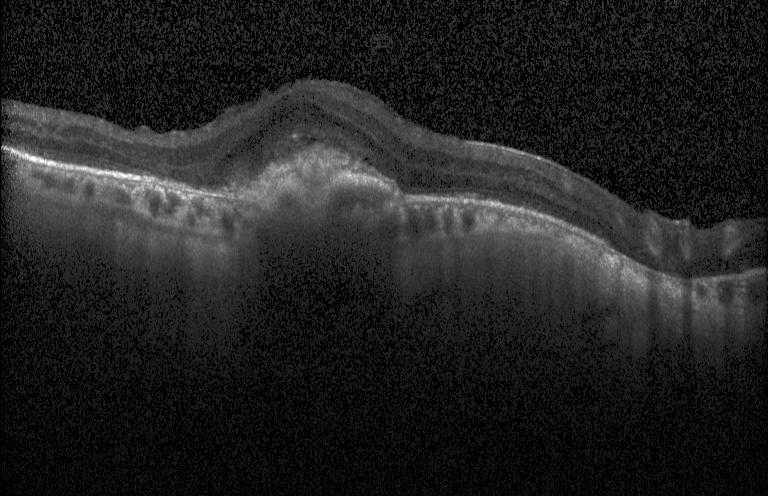
OCT finding: choroidal neovascularization (CNV).